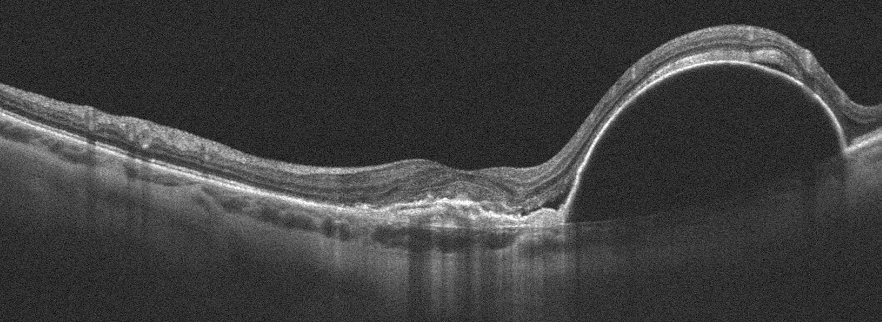
Retinal OCT B-scan. Acquired on an Optovue Avanti RTVue XR. Macular scan — Finding: AMD.